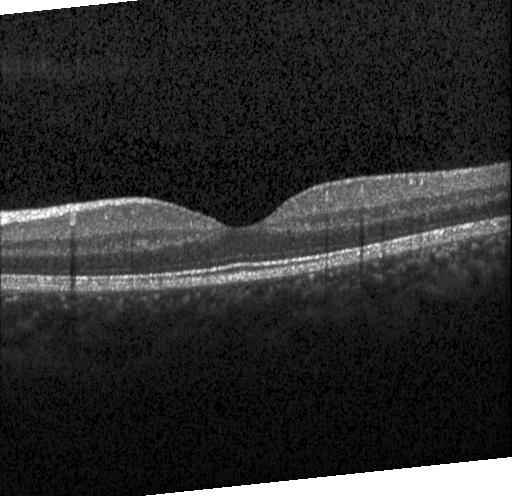 SD-OCT · optical coherence tomography B-scan · centered on the fovea
The scan shows neither CNV, DME, nor drusen.